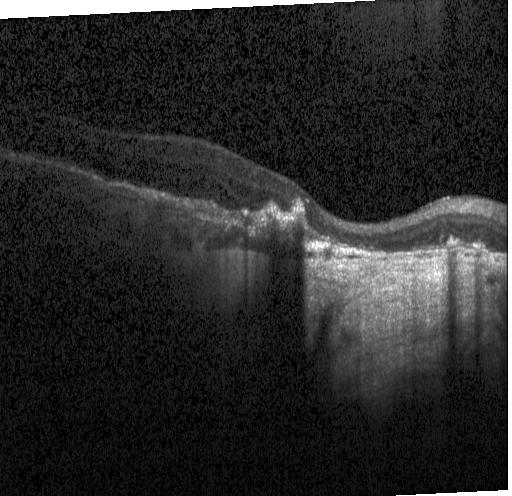

Optical coherence tomography B-scan.
Dx: choroidal neovascularization (CNV).